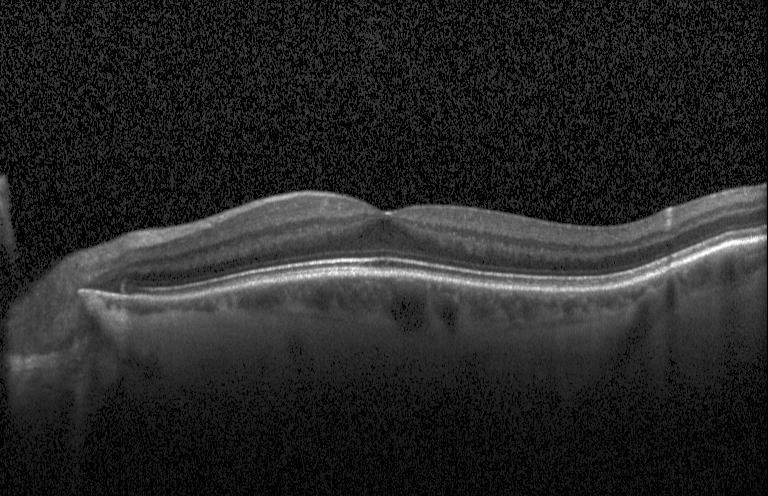
Instrument: Heidelberg Spectralis · retinal OCT B-scan. Assessment: neither choroidal neovascularization, diabetic macular edema, nor drusen.